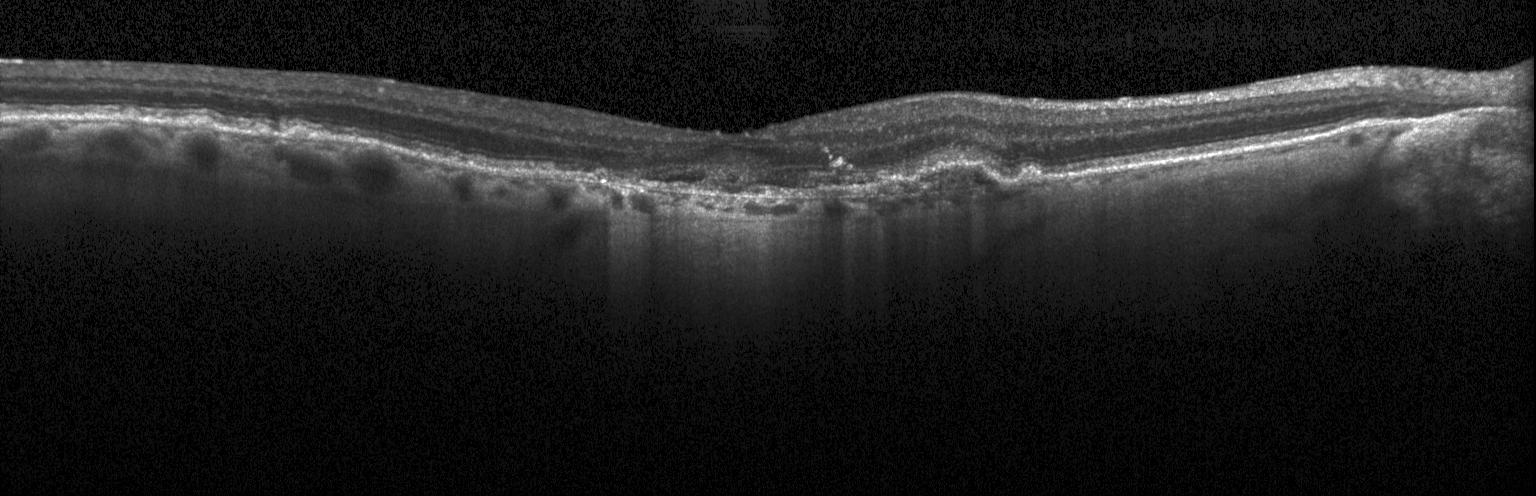 Heidelberg Spectralis OCT system; optical coherence tomography B-scan; SD-OCT
Dx: CNV.